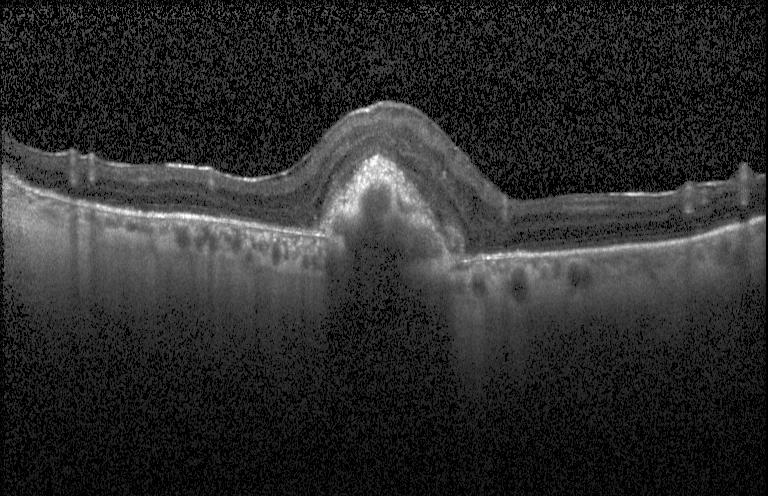 Optical coherence tomography B-scan · horizontal scan through the fovea
Macular OCT: choroidal neovascularization (CNV).